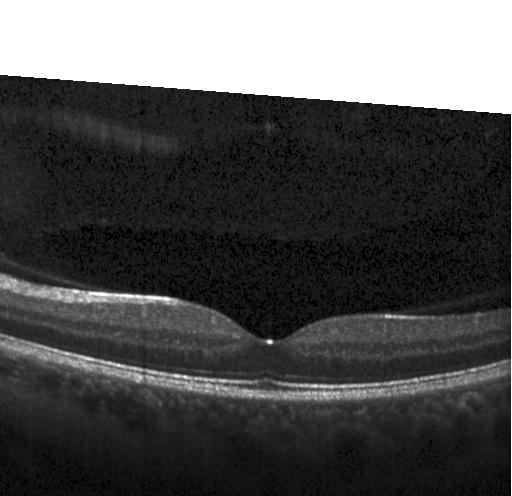
Retinal OCT B-scan; Heidelberg Spectralis OCT system.
Dx: no choroidal neovascularization, diabetic macular edema, or drusen.